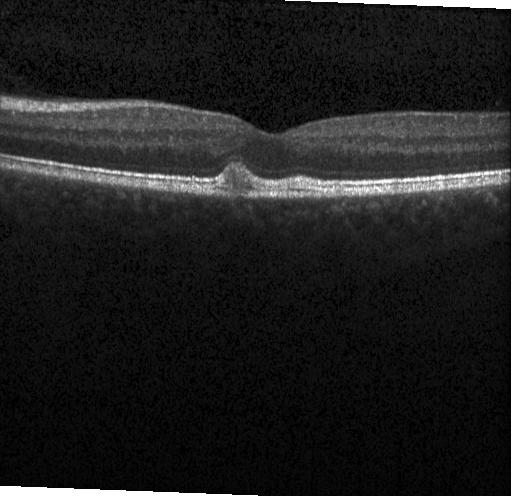

Optical coherence tomography B-scan. Spectral-domain optical coherence tomography. Heidelberg Spectralis. Macular scan.
The scan shows multiple drusen.